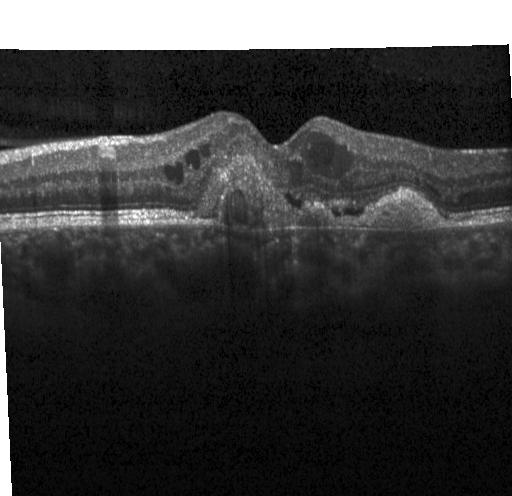

Retinal OCT cross-section
Macular OCT: choroidal neovascularization.